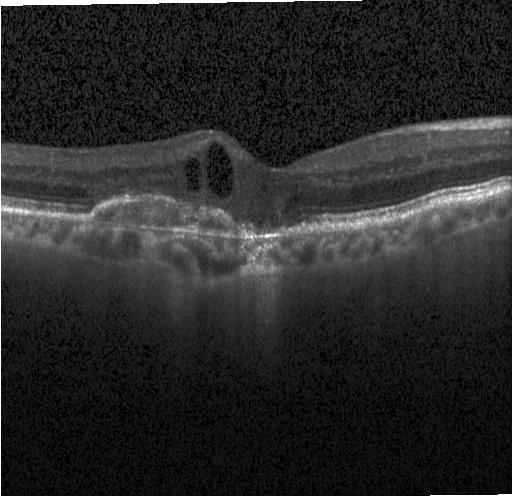
Heidelberg Spectralis. Optical coherence tomography B-scan.
The scan shows CNV.